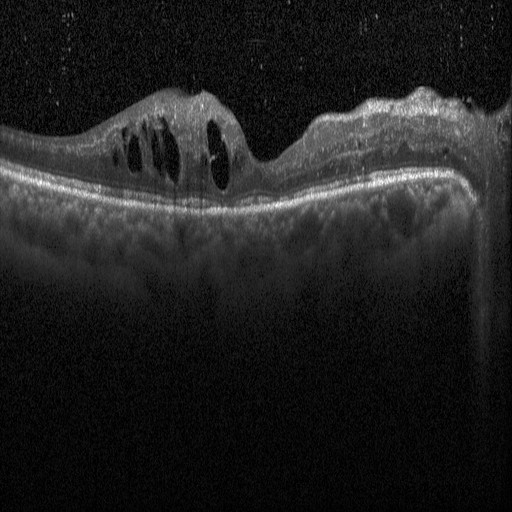 OCT line scan, spectral-domain optical coherence tomography, Heidelberg Spectralis OCT system.
Impression: diabetic macular edema.